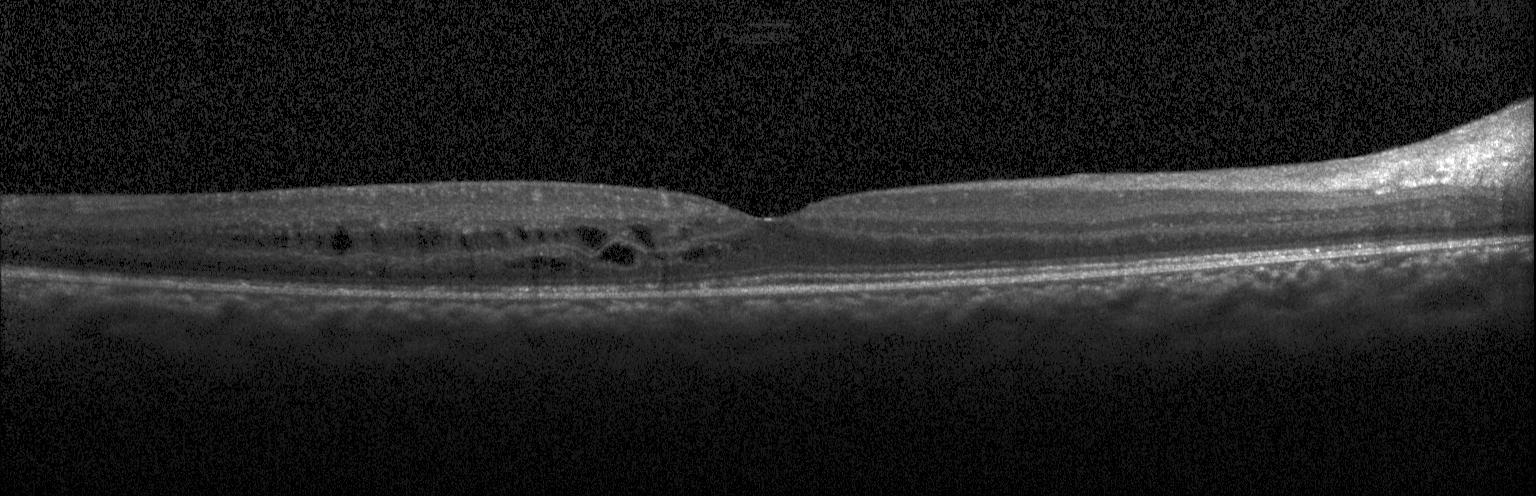

Heidelberg Spectralis. OCT B-scan. Assessment: DME.